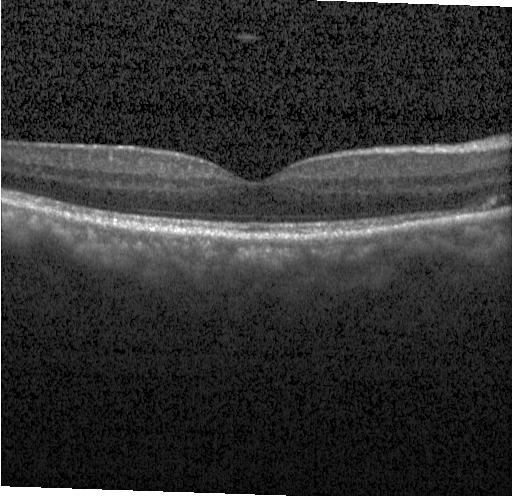

Assessment: no choroidal neovascularization, diabetic macular edema, or drusen.